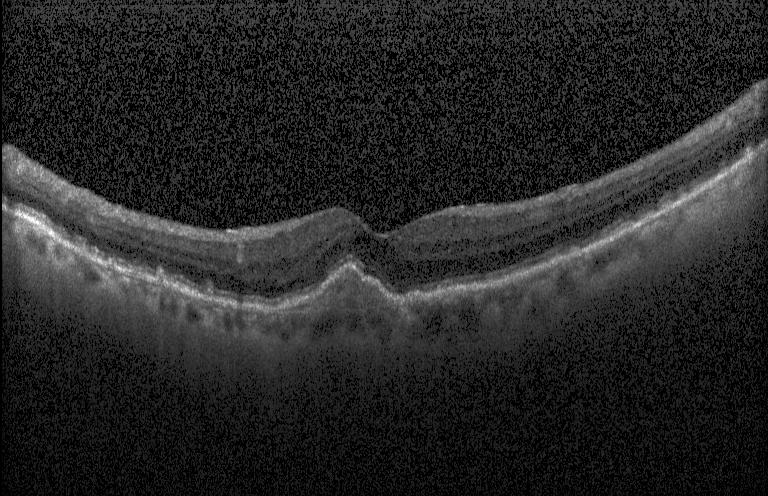 Optical coherence tomography B-scan. Macular scan. Finding: CNV.